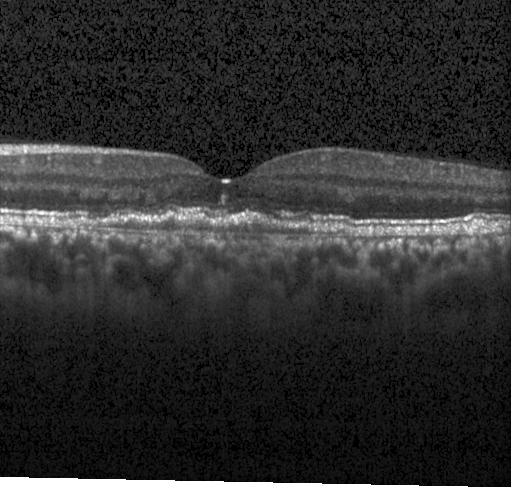
Macular OCT demonstrating choroidal neovascularization.